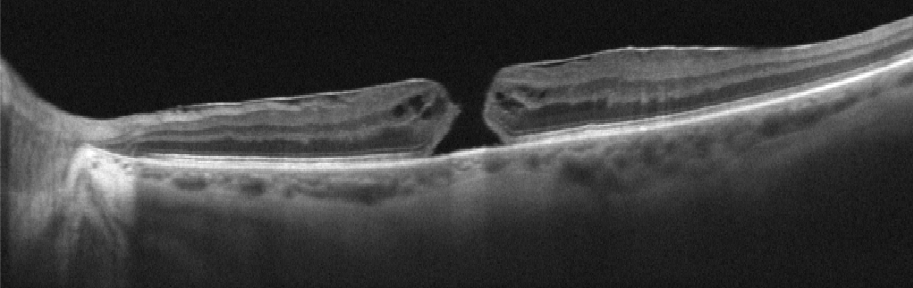

Retinal OCT cross-section. Fovea-centered — Finding: vitreomacular interface disease.